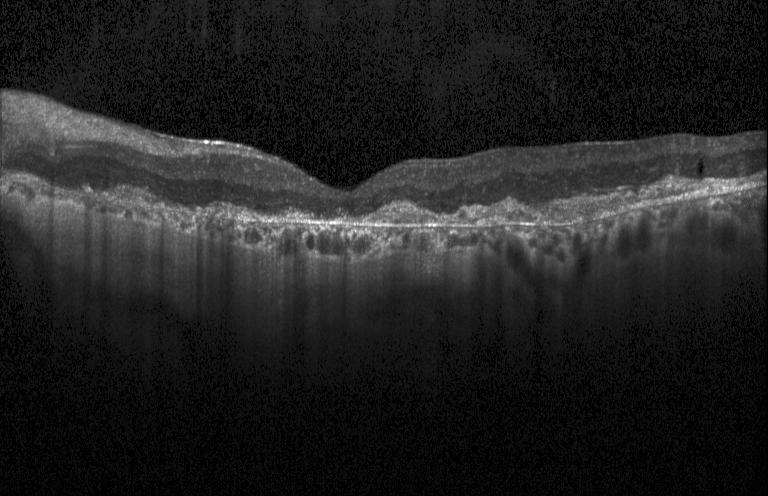
Optical coherence tomography scan. Diagnosis: a choroidal neovascular membrane.